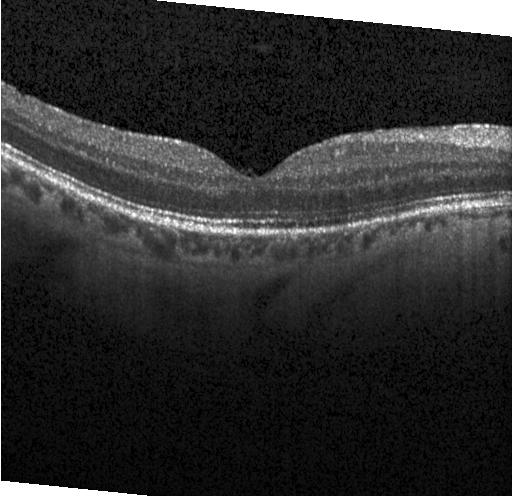
Optical coherence tomography B-scan
Macular OCT: neither choroidal neovascularization, diabetic macular edema, nor drusen.